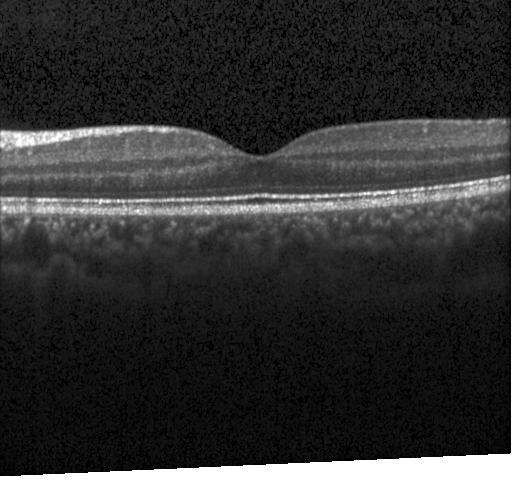

Instrument: Heidelberg Spectralis; SD-OCT; horizontal scan through the fovea; OCT B-scan — The scan shows no choroidal neovascularization, diabetic macular edema, or drusen.